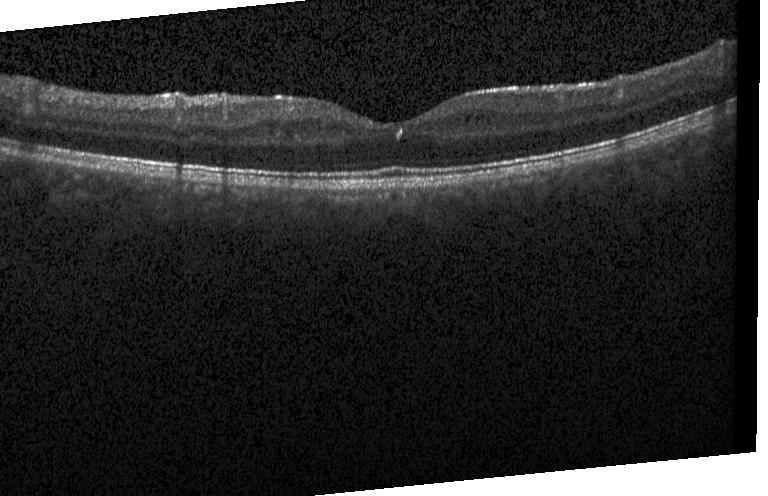 Dx: diabetic macular edema.